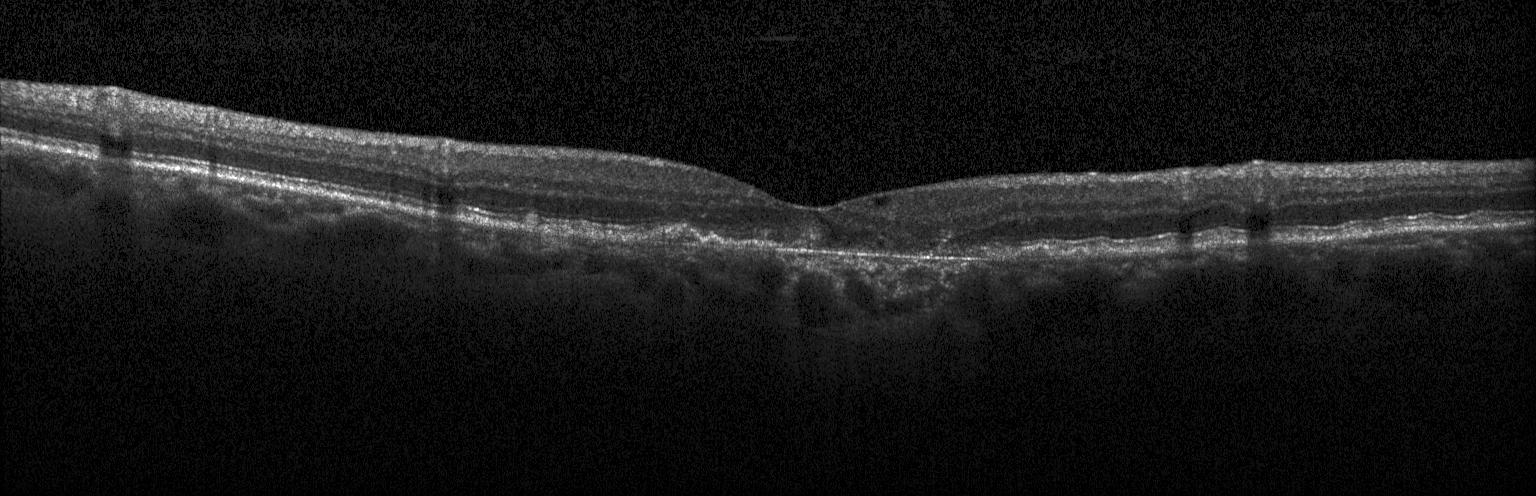
The scan shows a choroidal neovascular membrane.